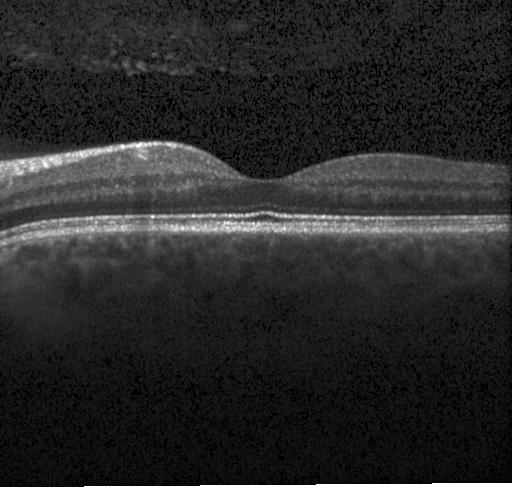
Retinal OCT B-scan. Finding: no choroidal neovascularization, diabetic macular edema, or drusen.